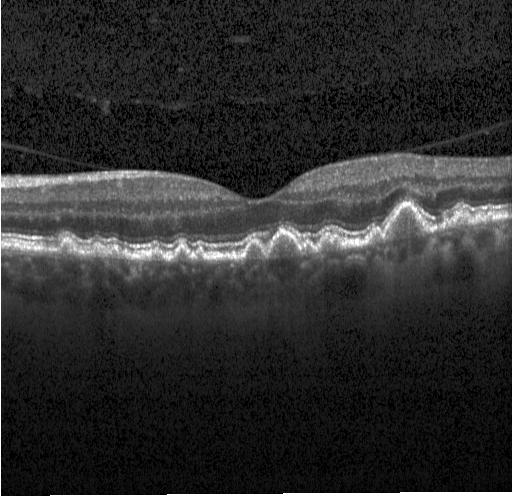
Optical coherence tomography scan — Dx: drusen.